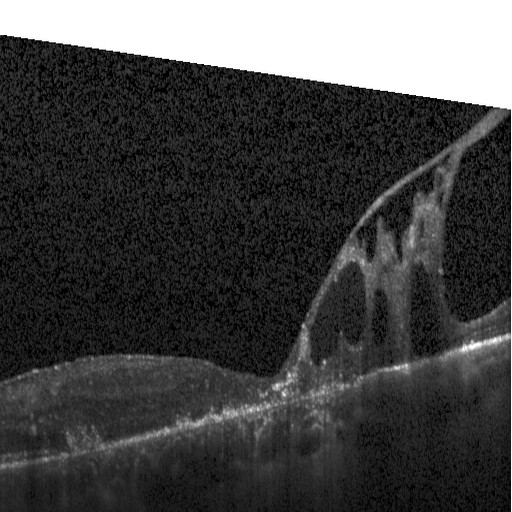 Macular OCT demonstrating diabetic macular edema.